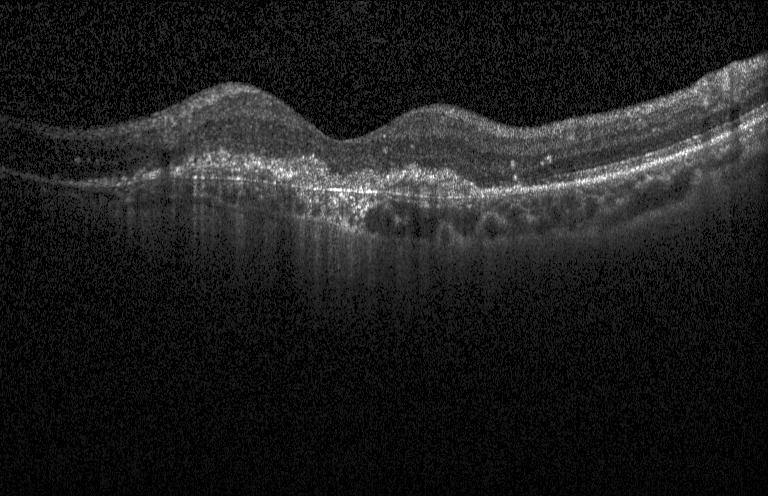
Spectral-domain OCT B-scan: CNV.